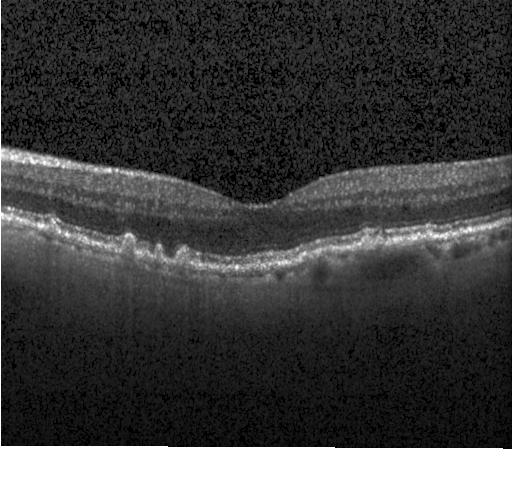
Retinal OCT cross-section; through the macula
Assessment: drusen.